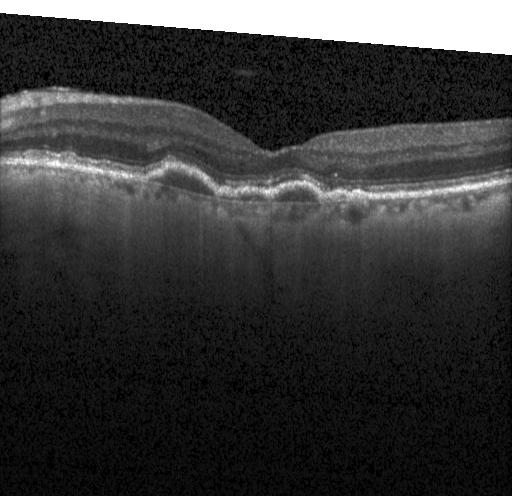
Spectral-domain OCT B-scan: CNV.